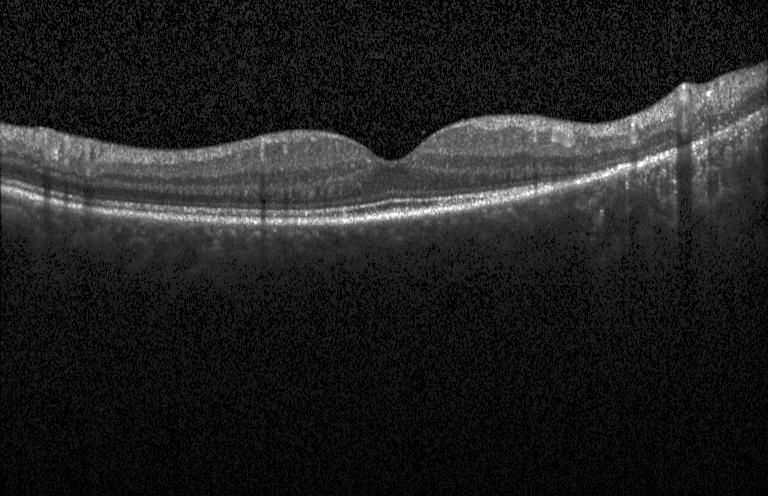

No evidence of choroidal neovascularization, diabetic macular edema, or drusen.